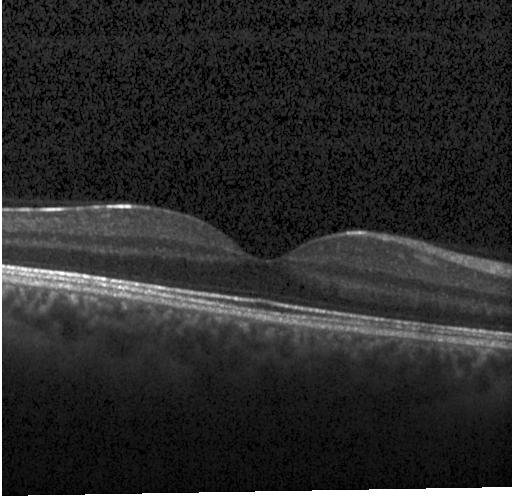
OCT finding: no choroidal neovascularization, diabetic macular edema, or drusen.